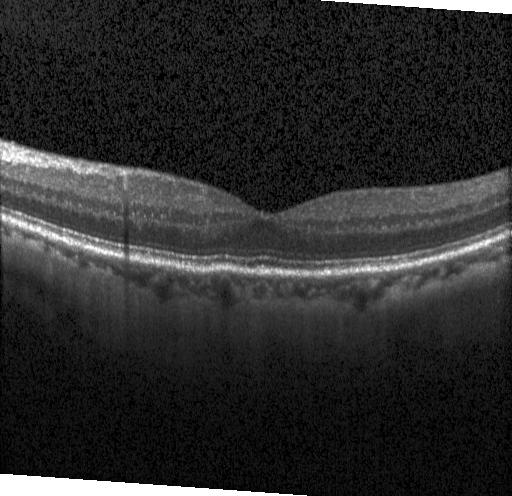
Heidelberg Spectralis; horizontal scan through the fovea; optical coherence tomography B-scan; SD-OCT. No evidence of CNV, DME, or drusen.